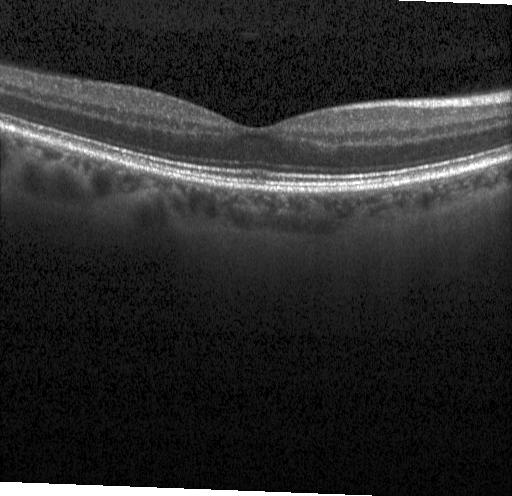 Heidelberg Spectralis OCT system · optical coherence tomography scan · SD-OCT · through the macula.
Dx: no choroidal neovascularization, diabetic macular edema, or drusen.